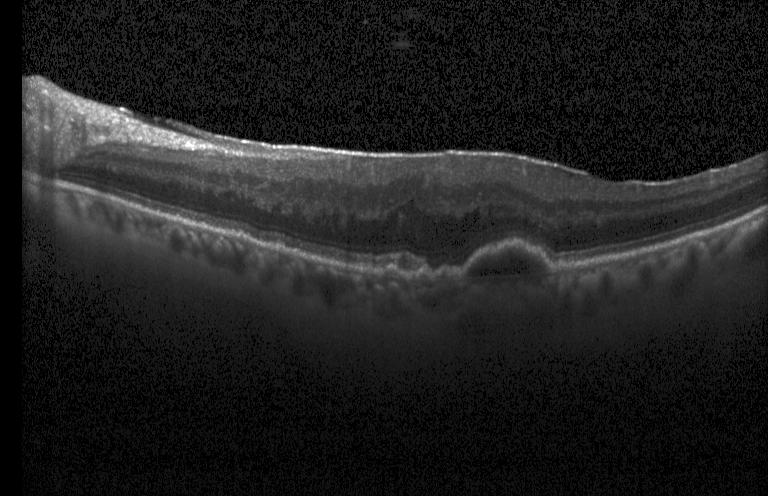 OCT B-scan.
OCT finding: choroidal neovascularization (CNV).